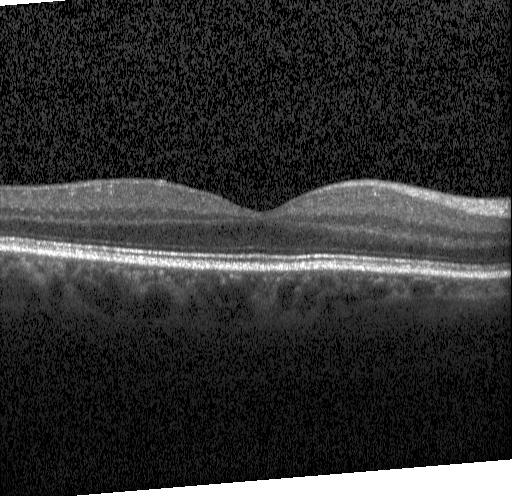
Retinal OCT B-scan. Diagnosis: no choroidal neovascularization, no diabetic macular edema, and no drusen.